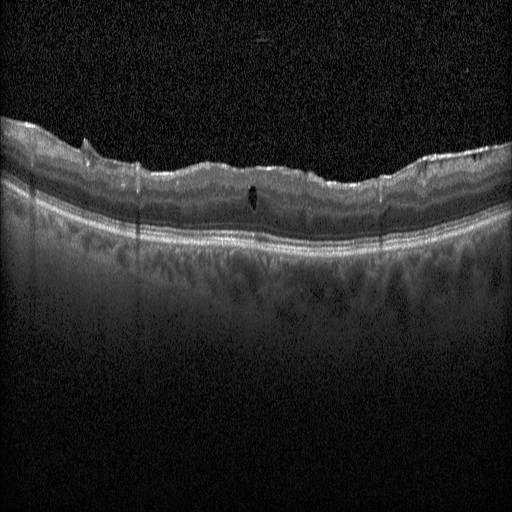 Diagnosis: diabetic macular edema (DME).